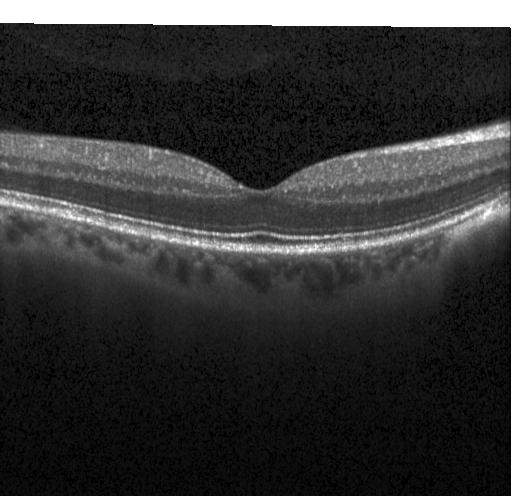

OCT line scan. Diagnosis: no choroidal neovascularization, no diabetic macular edema, and no drusen.